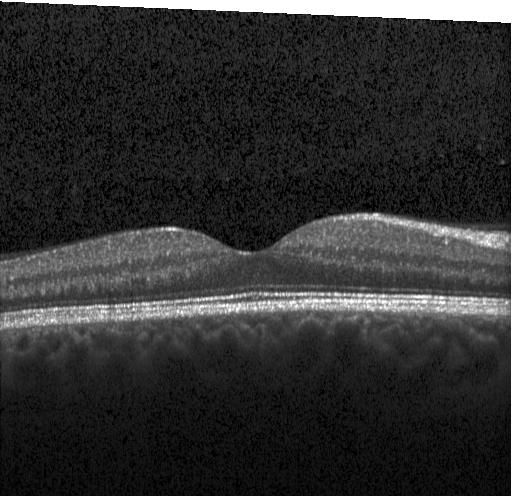

Acquired on a Heidelberg Spectralis, OCT B-scan
Finding: neither choroidal neovascularization, diabetic macular edema, nor drusen.